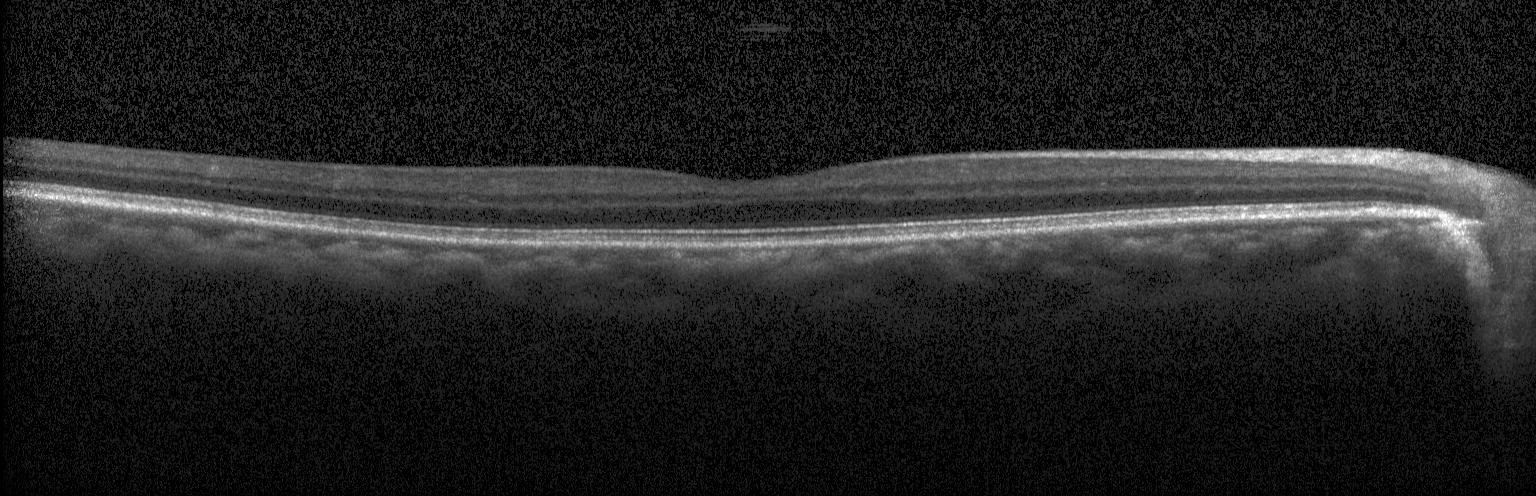 Retinal OCT cross-section. Impression: no choroidal neovascularization, no diabetic macular edema, and no drusen.